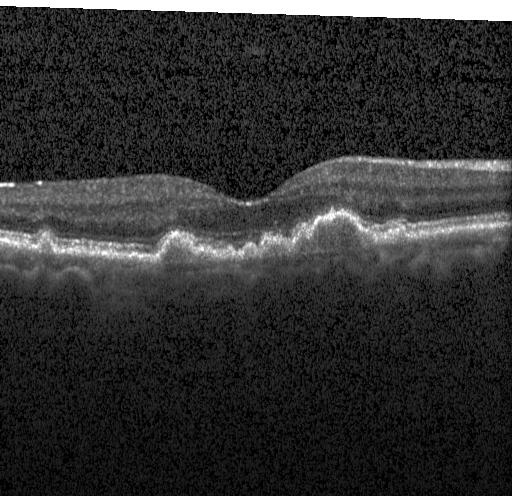 Macular scan. Spectral-domain OCT. Optical coherence tomography scan. Acquired on a Heidelberg Spectralis.
The scan shows multiple drusen.